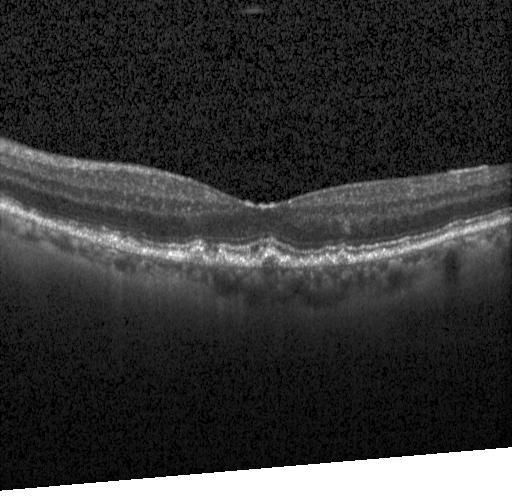

Retinal OCT cross-section showing multiple drusen.